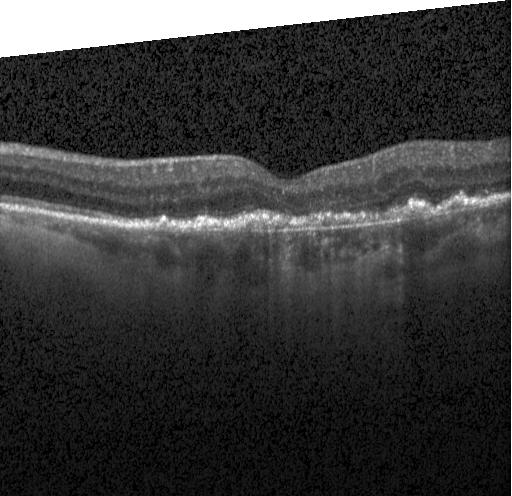

Spectral-domain optical coherence tomography · instrument: Heidelberg Spectralis · OCT B-scan · macular scan
Diagnosis: CNV.